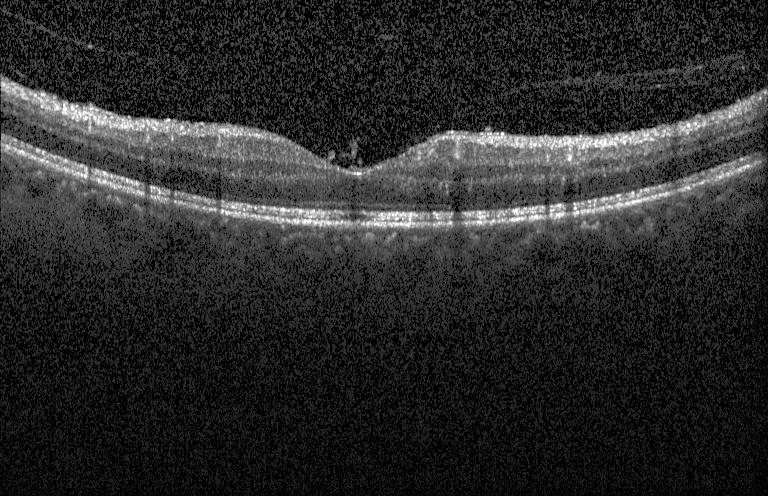

SD-OCT · instrument: Heidelberg Spectralis · macular scan · OCT line scan
OCT finding: no CNV, no DME, and no drusen.